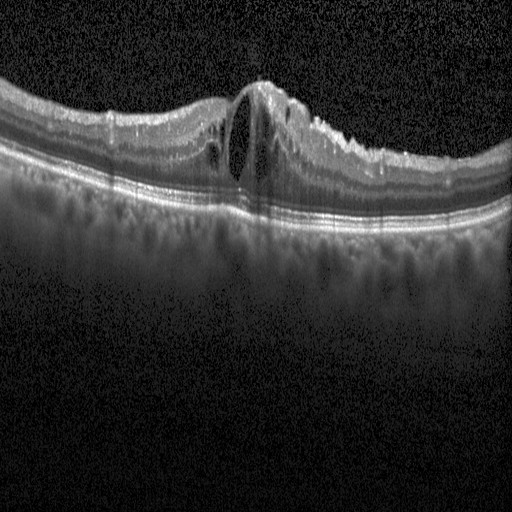
Impression: diabetic macular edema.